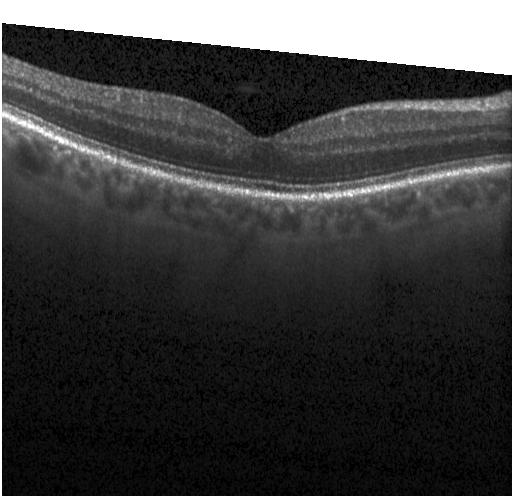
Optical coherence tomography scan; spectral-domain OCT; instrument: Heidelberg Spectralis; through the macula — Assessment: no choroidal neovascularization, diabetic macular edema, or drusen.